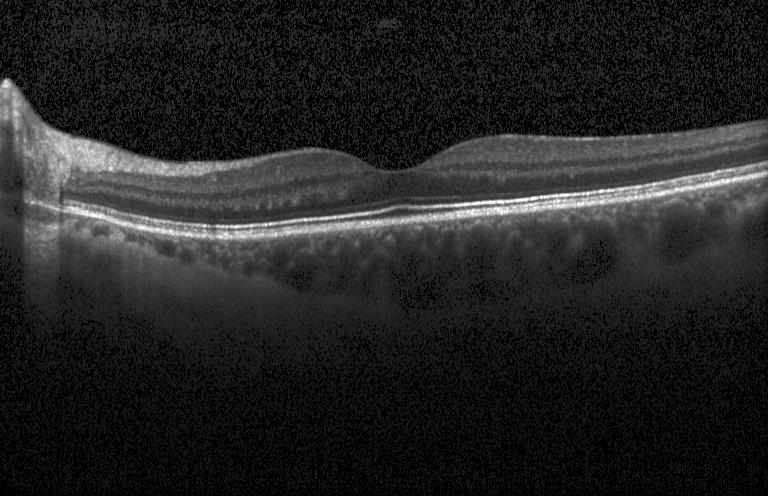 Optical coherence tomography scan.
Finding: neither choroidal neovascularization, diabetic macular edema, nor drusen.